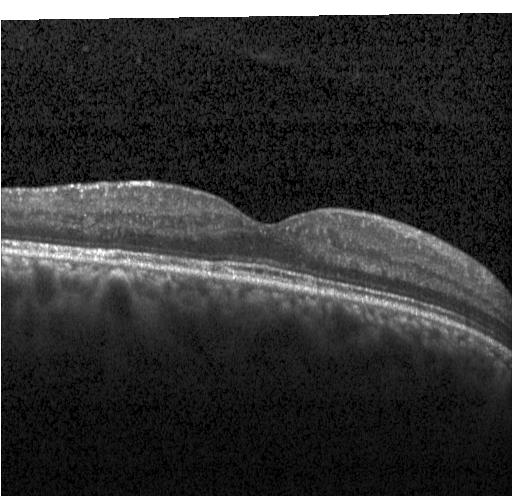

OCT B-scan — OCT finding: neither choroidal neovascularization, diabetic macular edema, nor drusen.